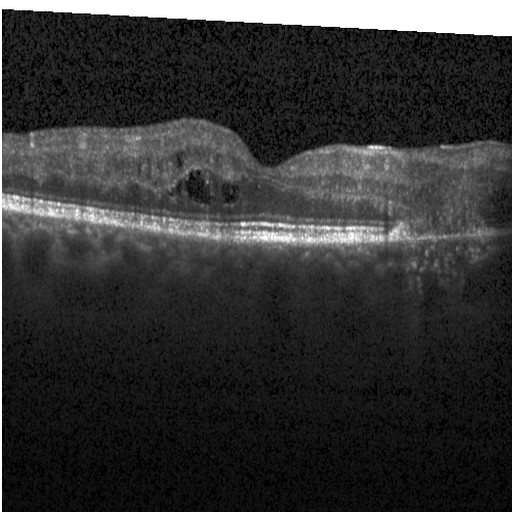

Retinal OCT cross-section, centered on the fovea, Heidelberg Spectralis OCT system, spectral-domain optical coherence tomography.
Impression: diabetic macular edema.